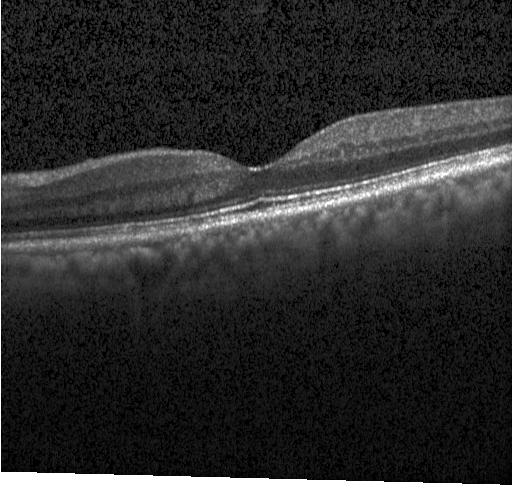

OCT line scan
OCT finding: neither choroidal neovascularization, diabetic macular edema, nor drusen.